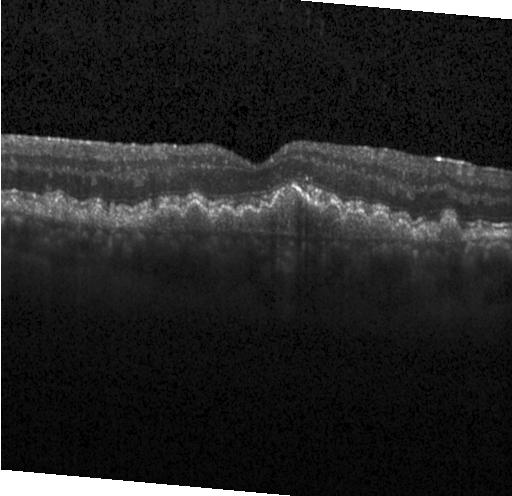 Impression: a choroidal neovascular membrane.